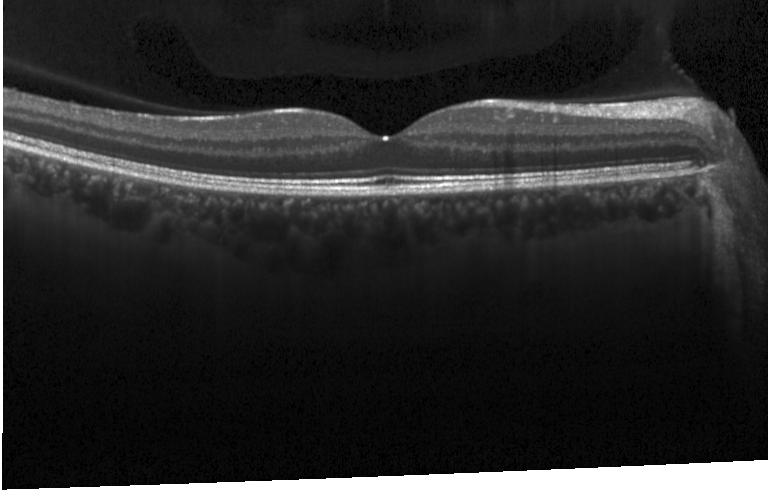

Optical coherence tomography scan — Assessment: no CNV, no DME, and no drusen.